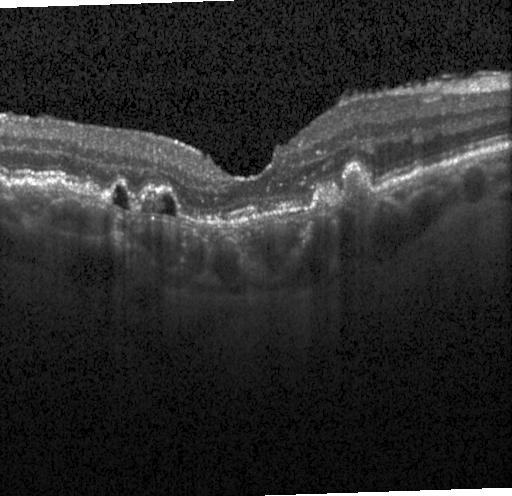
Through the macula, OCT line scan, SD-OCT.
Diagnosis: a choroidal neovascular membrane.